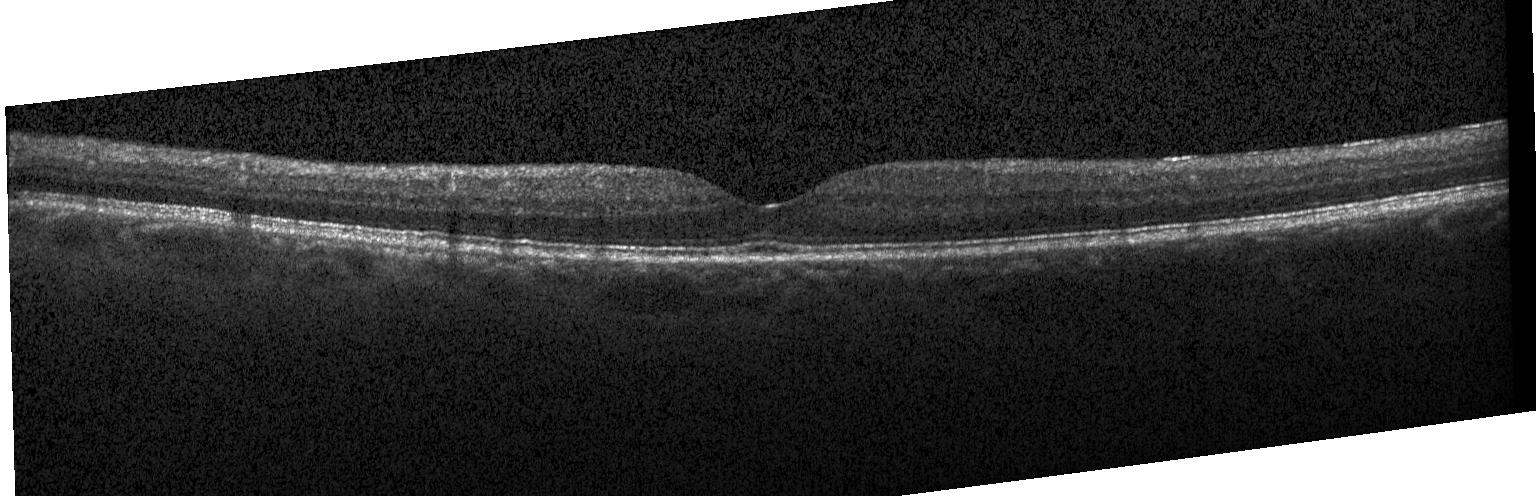 Optical coherence tomography scan.
Diagnosis: no choroidal neovascularization, diabetic macular edema, or drusen.